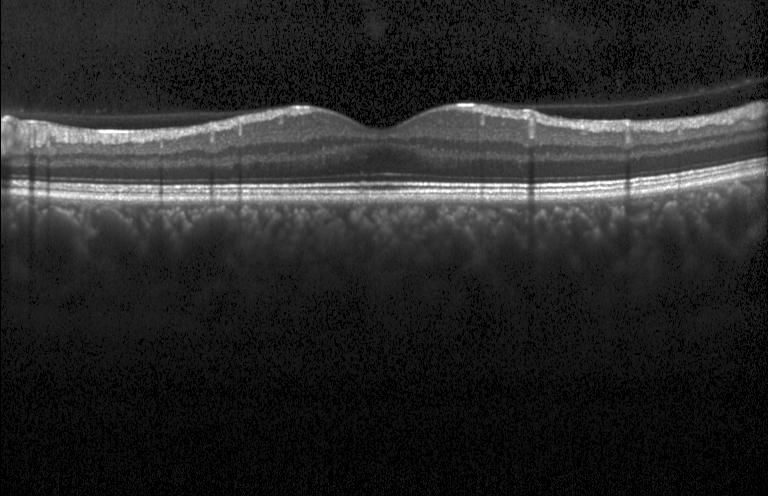 Retinal OCT B-scan; instrument: Heidelberg Spectralis; spectral-domain optical coherence tomography
Impression: no choroidal neovascularization, diabetic macular edema, or drusen.